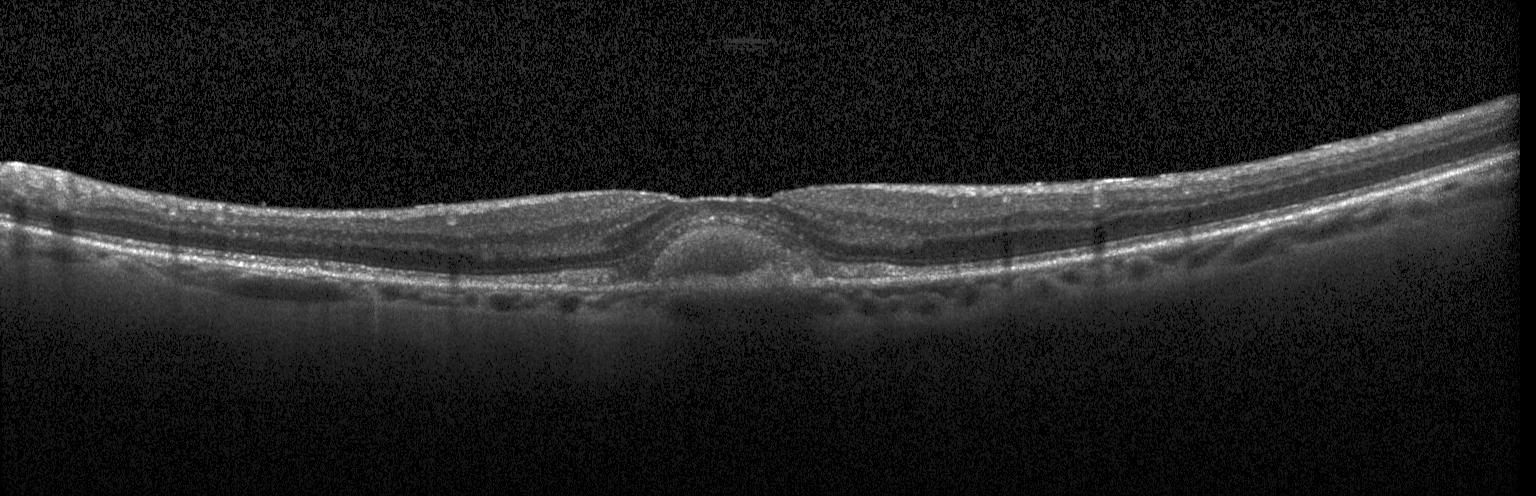

Diagnosis: choroidal neovascularization.